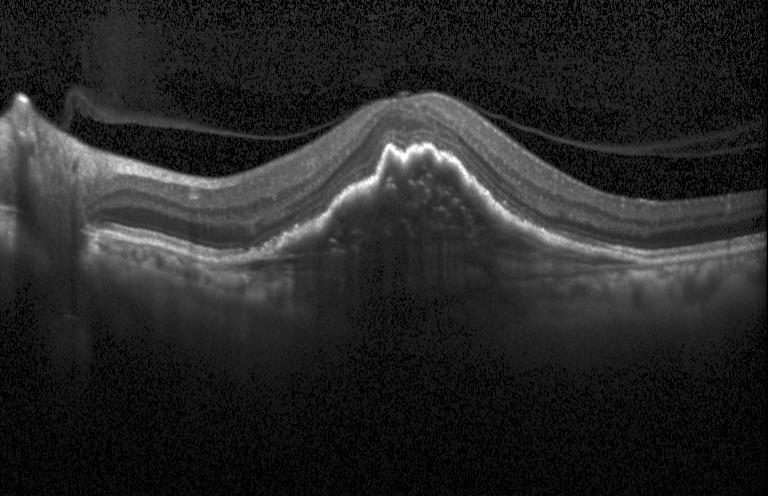
Optical coherence tomography B-scan
Finding: a choroidal neovascular membrane.